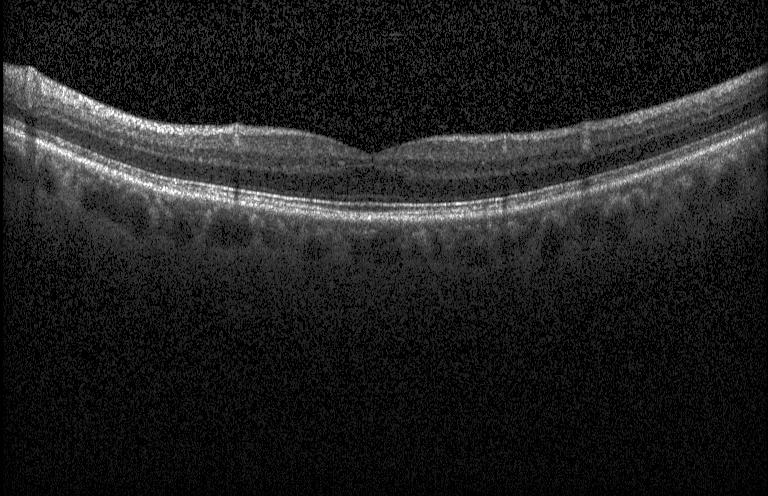
Retinal OCT cross-section showing no CNV, no DME, and no drusen.